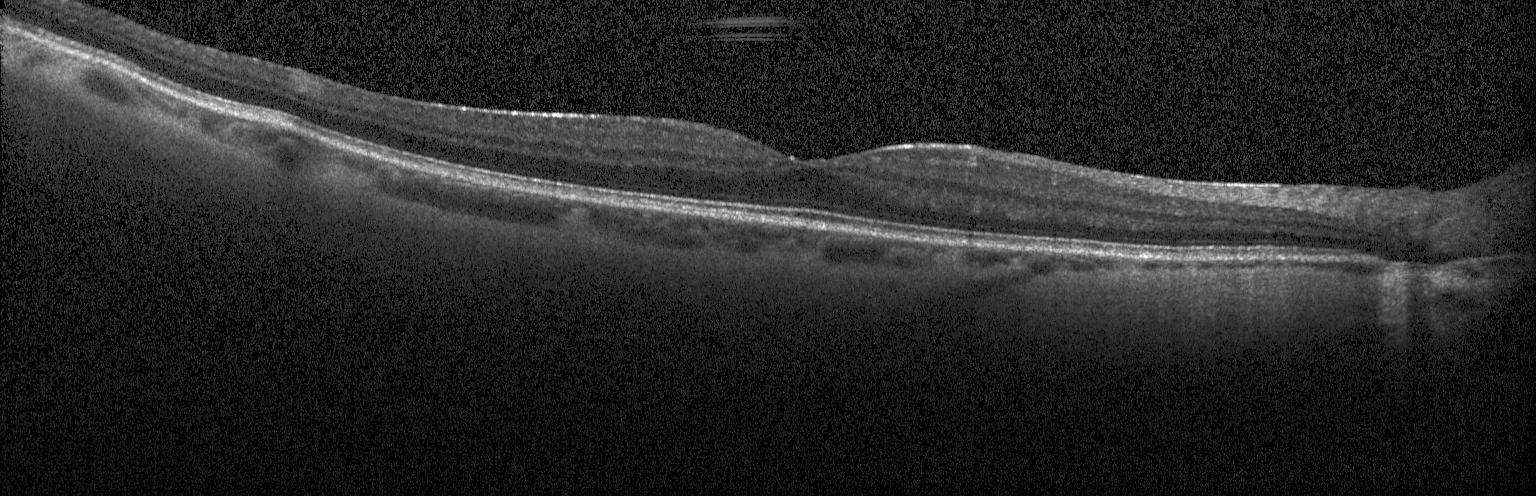

Fovea-centered; OCT B-scan — Dx: no choroidal neovascularization, no diabetic macular edema, and no drusen.